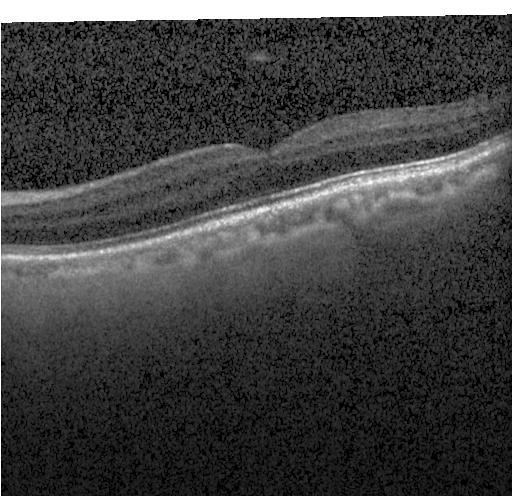 Diagnosis: no choroidal neovascularization, diabetic macular edema, or drusen.